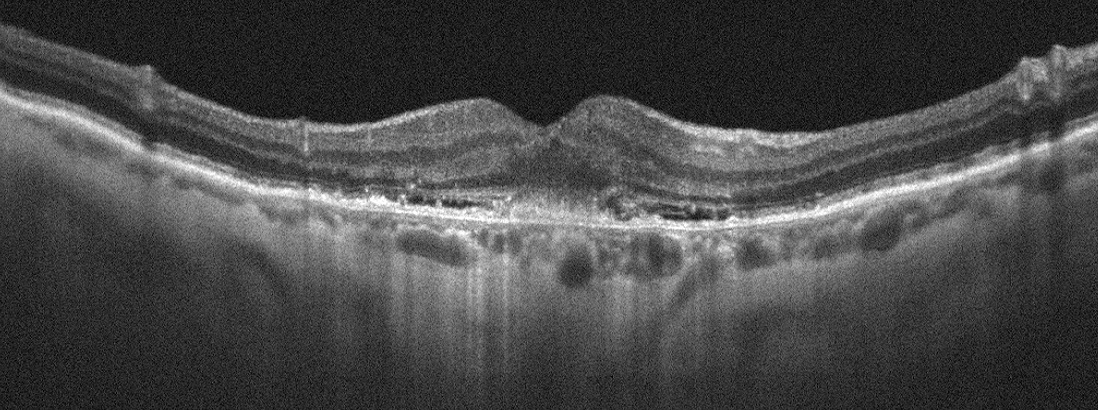

Acquired on an Optovue Avanti RTVue XR; OCT B-scan; macular scan. Age-related macular degeneration (AMD).